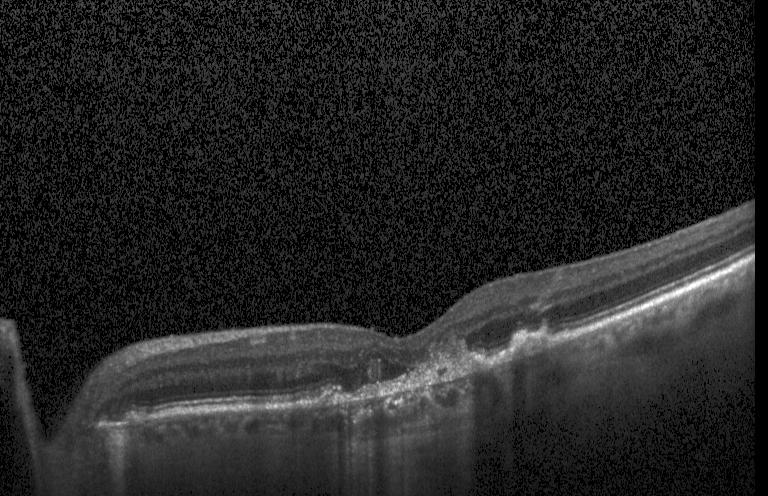
OCT line scan — Finding: a choroidal neovascular membrane.